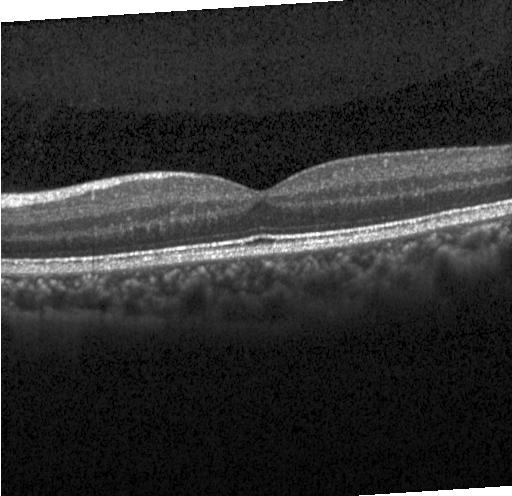
Optical coherence tomography scan. Spectral-domain OCT. Instrument: Heidelberg Spectralis. Centered on the fovea.
Assessment: neither CNV, DME, nor drusen.